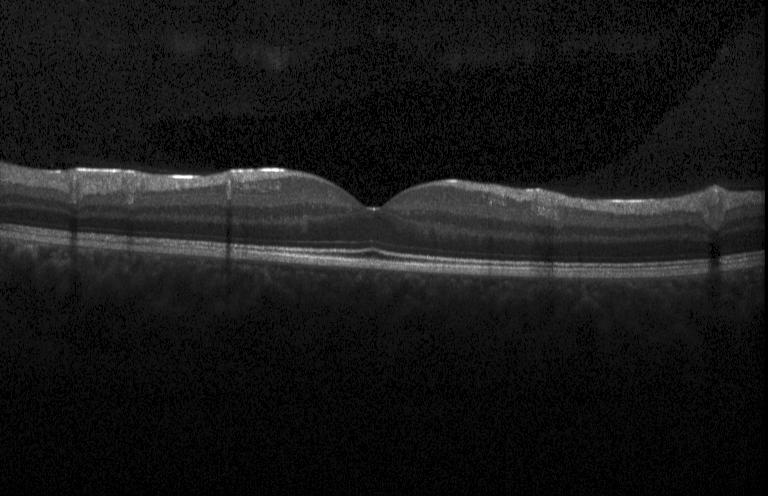
Macular OCT demonstrating no choroidal neovascularization, no diabetic macular edema, and no drusen.